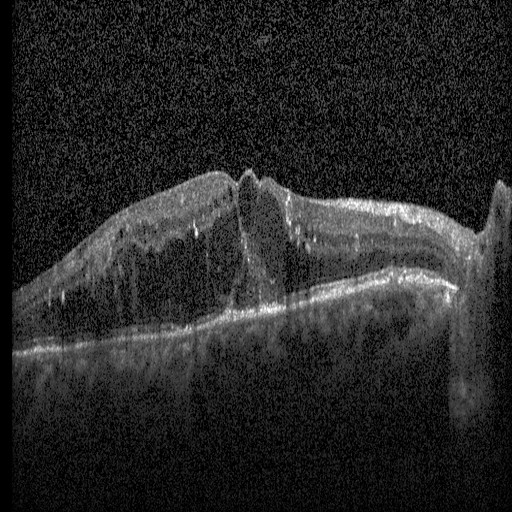 Retinal OCT B-scan; centered on the fovea; spectral-domain OCT. Assessment: diabetic macular edema (DME).